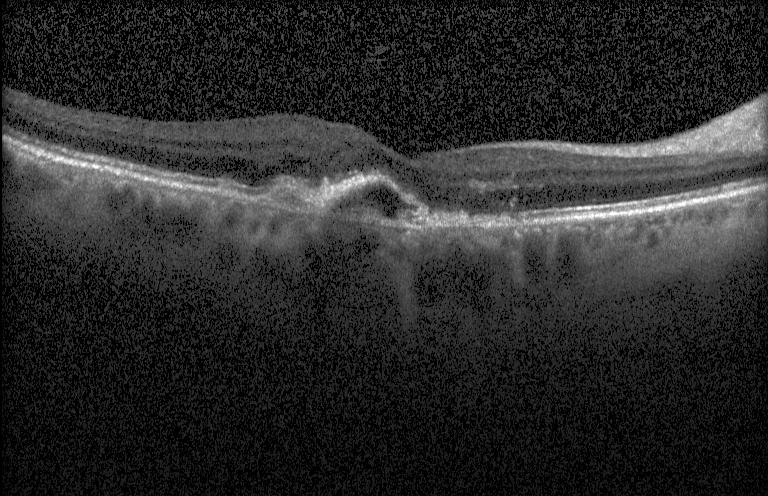
Dx: choroidal neovascularization (CNV).